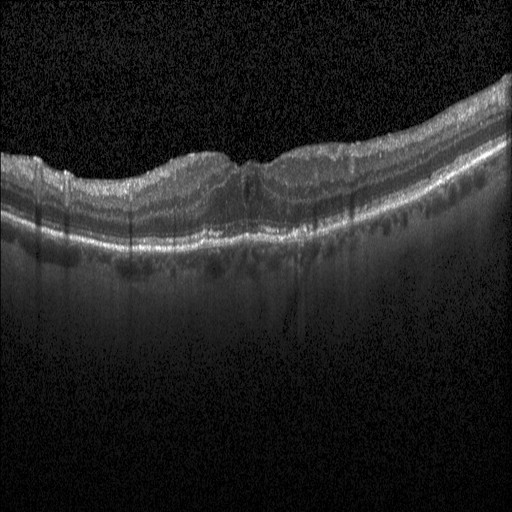

Fovea-centered · spectral-domain optical coherence tomography · OCT line scan.
Finding: DME.